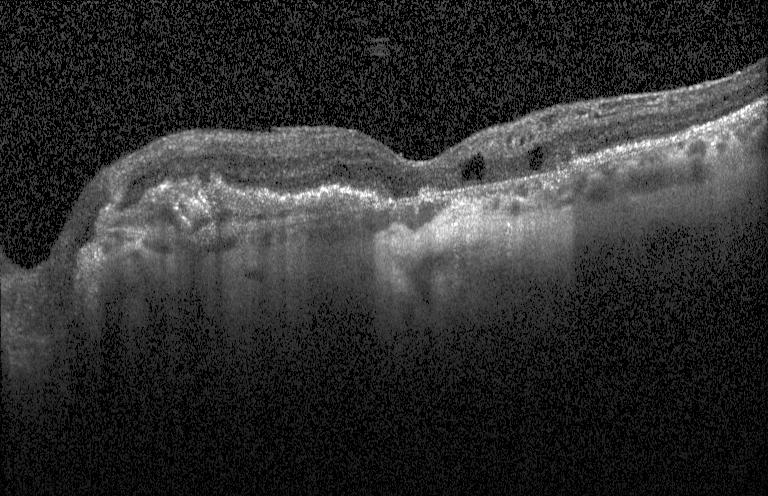
Fovea-centered · optical coherence tomography B-scan · SD-OCT · Heidelberg Spectralis OCT system
Assessment: choroidal neovascularization (CNV).